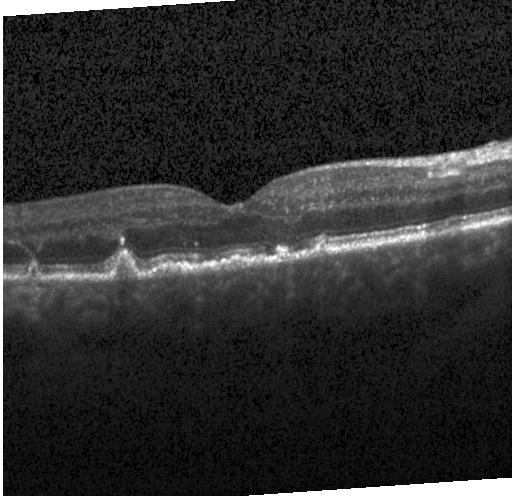 Diagnosis: multiple drusen.